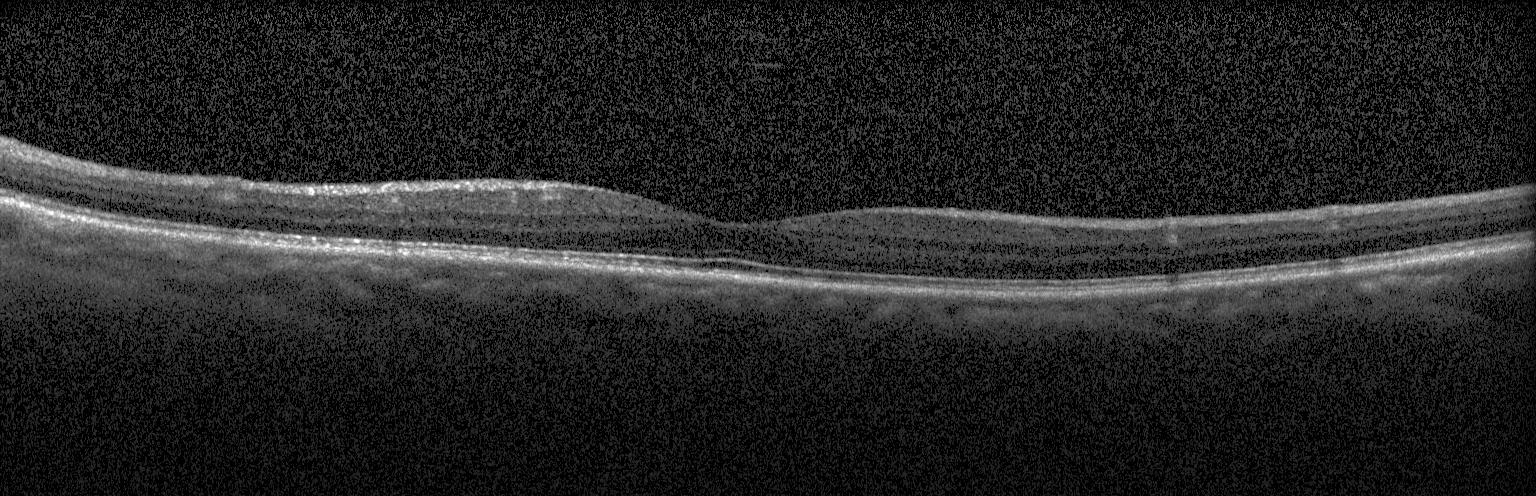

Macular OCT demonstrating no evidence of CNV, DME, or drusen.